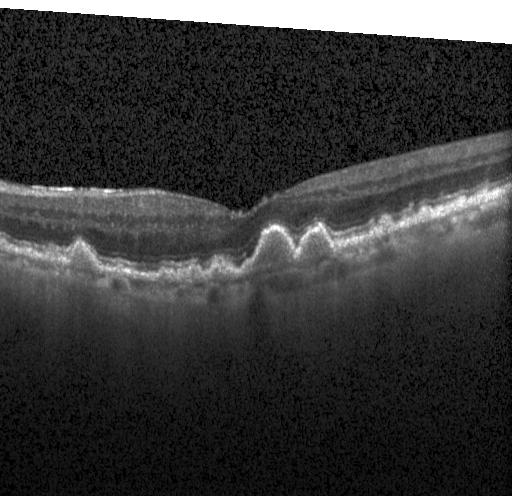
Macular scan; spectral-domain OCT; instrument: Heidelberg Spectralis; OCT line scan — Sub-RPE drusenoid deposits.